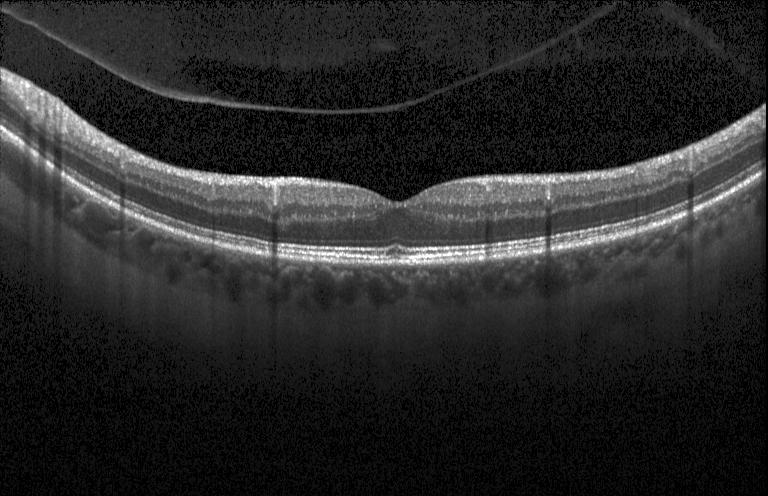 OCT B-scan. Acquired on a Heidelberg Spectralis. Macular scan. SD-OCT
Impression: no evidence of choroidal neovascularization, diabetic macular edema, or drusen.